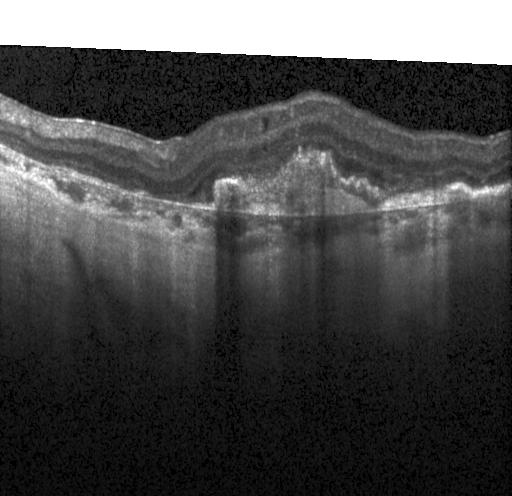 Diagnosis: choroidal neovascularization (CNV).